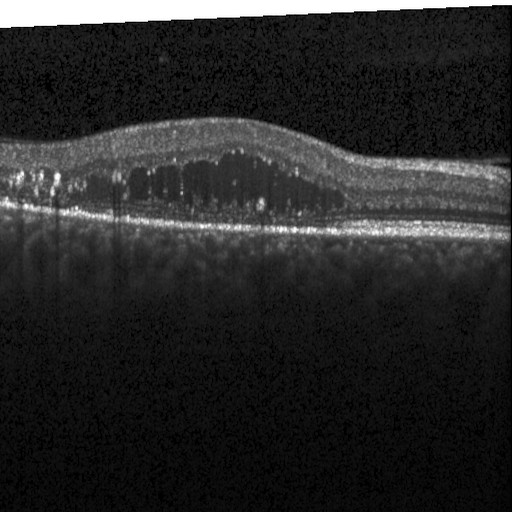
SD-OCT, horizontal scan through the fovea, OCT line scan, acquired on a Heidelberg Spectralis — This B-scan demonstrates diabetic macular edema (DME).